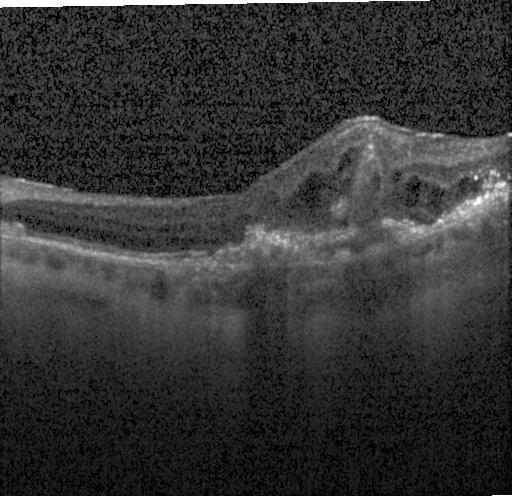
Diagnosis: a choroidal neovascular membrane.